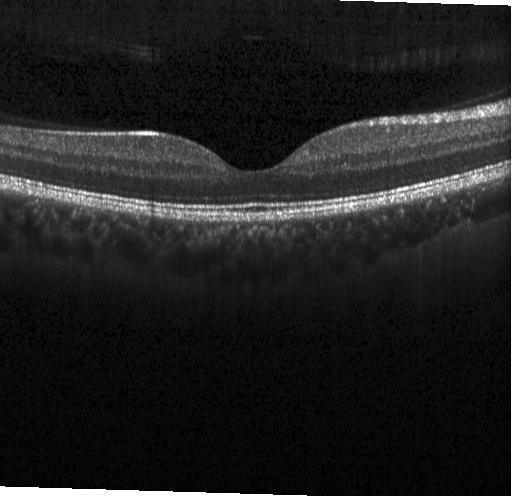
Dx: neither choroidal neovascularization, diabetic macular edema, nor drusen.